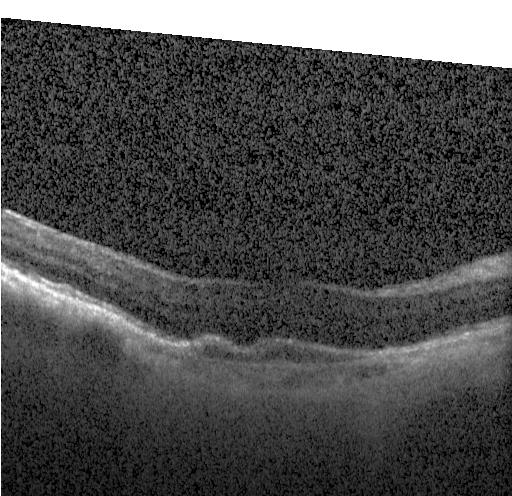
OCT B-scan showing choroidal neovascularization (CNV).